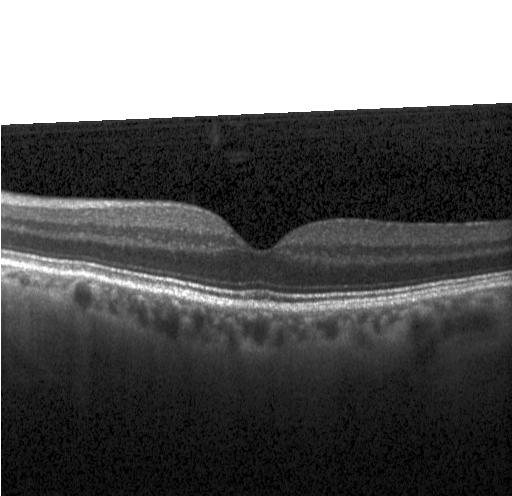 Macular scan. Spectral-domain optical coherence tomography. Instrument: Heidelberg Spectralis. Optical coherence tomography scan.
Impression: no evidence of choroidal neovascularization, diabetic macular edema, or drusen.